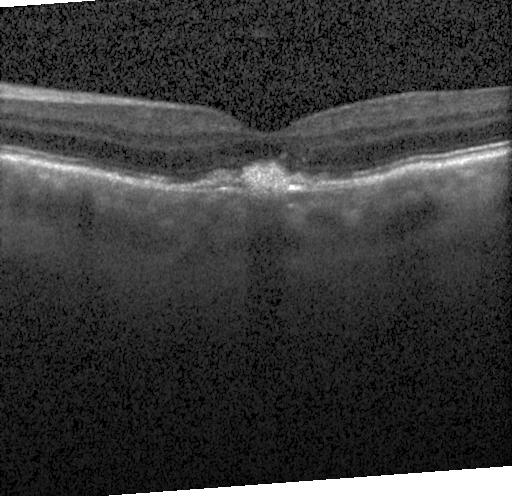

Retinal OCT cross-section.
Finding: choroidal neovascularization (CNV).